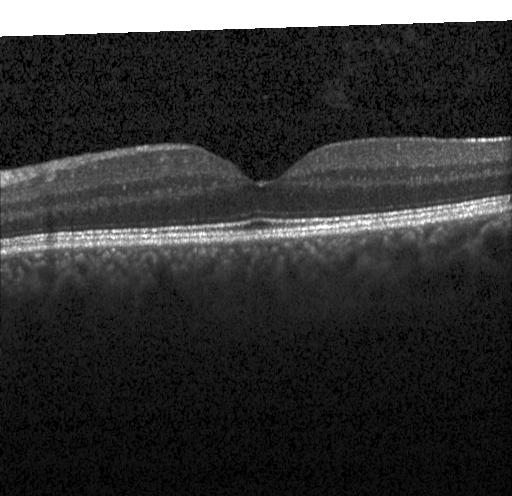

The scan shows no evidence of choroidal neovascularization, diabetic macular edema, or drusen.